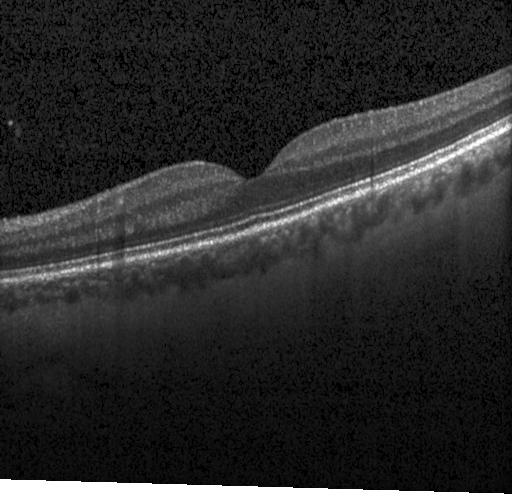
SD-OCT, retinal OCT cross-section, macular scan. This B-scan demonstrates no choroidal neovascularization, diabetic macular edema, or drusen.